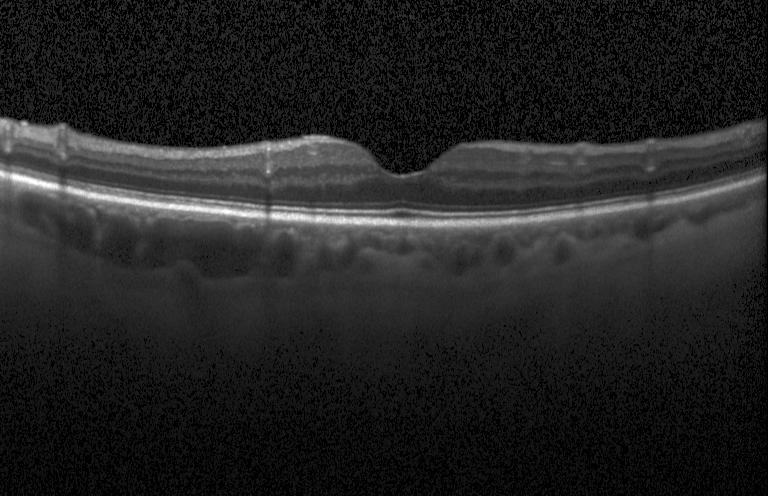 OCT finding: neither choroidal neovascularization, diabetic macular edema, nor drusen.